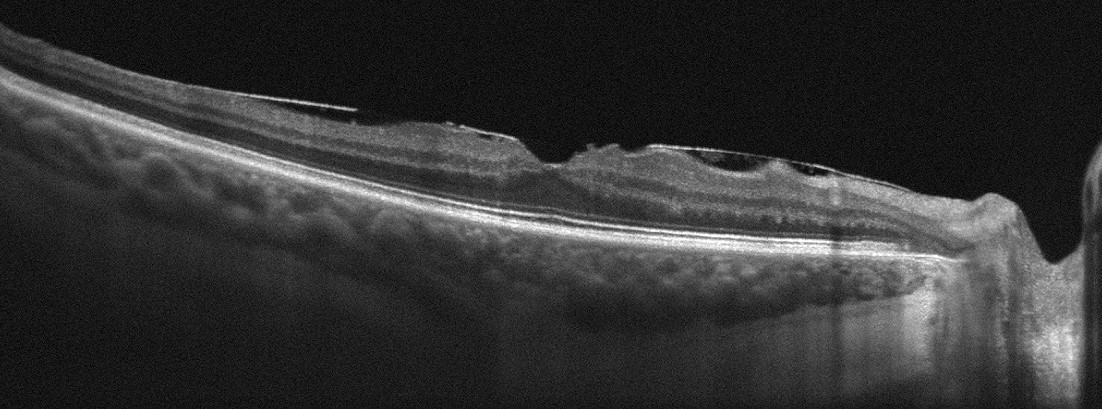

Optical coherence tomography scan — Macular OCT: epiretinal membrane (ERM).